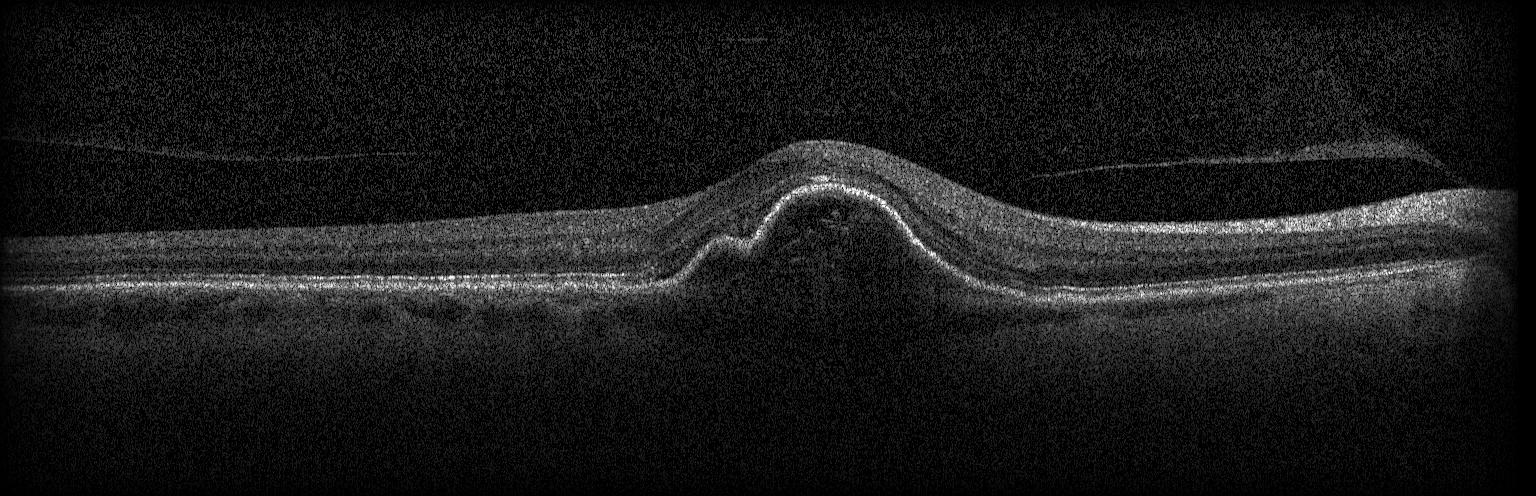 Retinal OCT B-scan. Acquired on a Heidelberg Spectralis.
Impression: CNV.